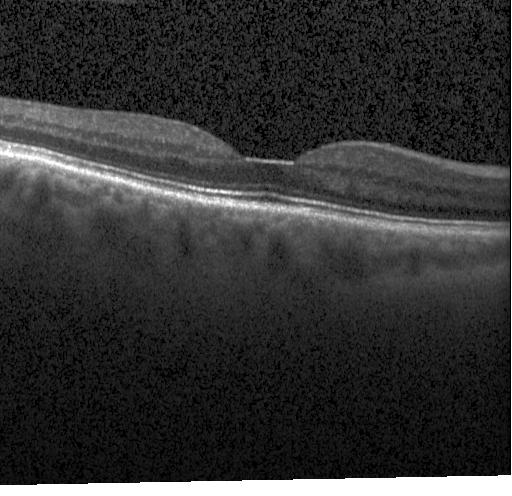

The scan shows no CNV, no DME, and no drusen.